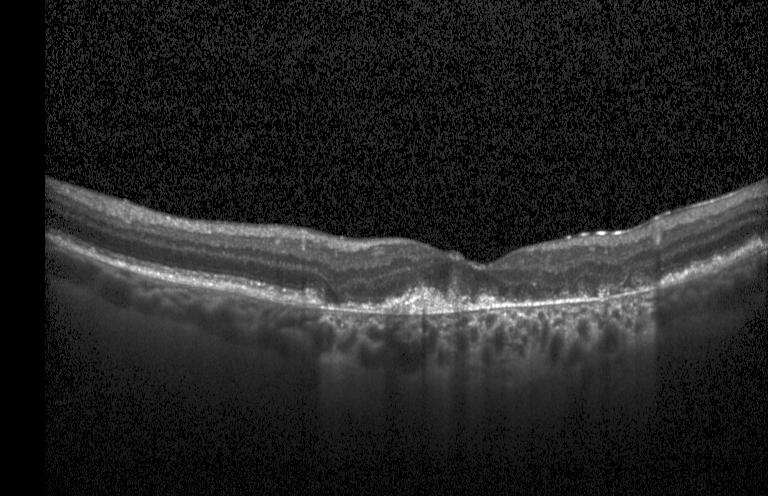 Through the macula; OCT B-scan; SD-OCT — OCT finding: a choroidal neovascular membrane.